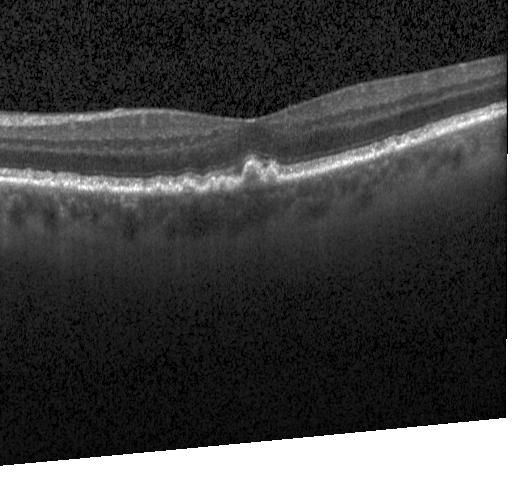 Retinal OCT cross-section showing drusen.